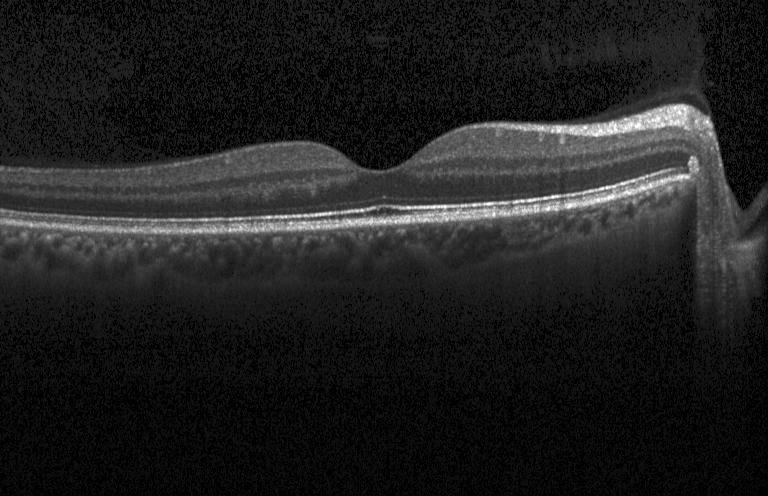

Spectral-domain optical coherence tomography. Fovea-centered. OCT line scan
Assessment: no evidence of CNV, DME, or drusen.